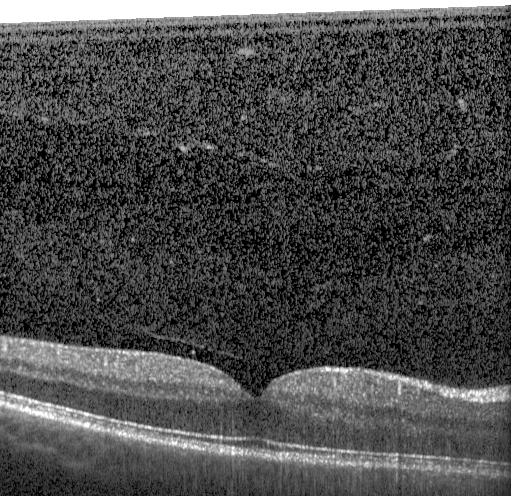

Macular scan · acquired on a Heidelberg Spectralis · optical coherence tomography scan · spectral-domain optical coherence tomography.
Impression: no evidence of choroidal neovascularization, diabetic macular edema, or drusen.